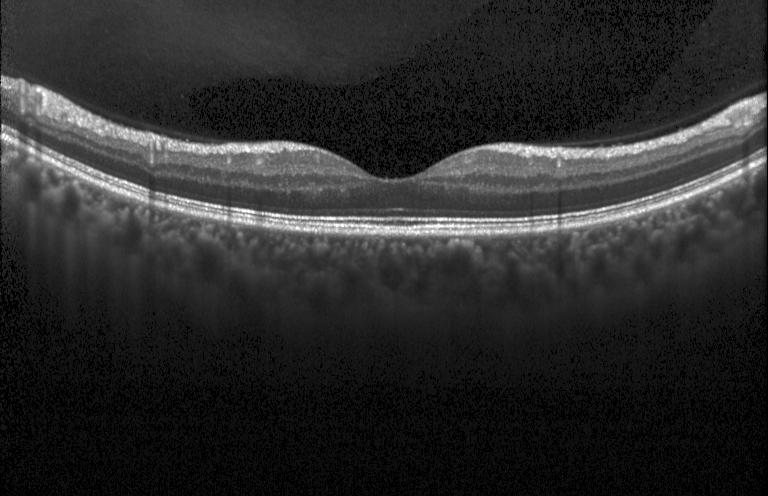 OCT B-scan. SD-OCT — Finding: neither CNV, DME, nor drusen.